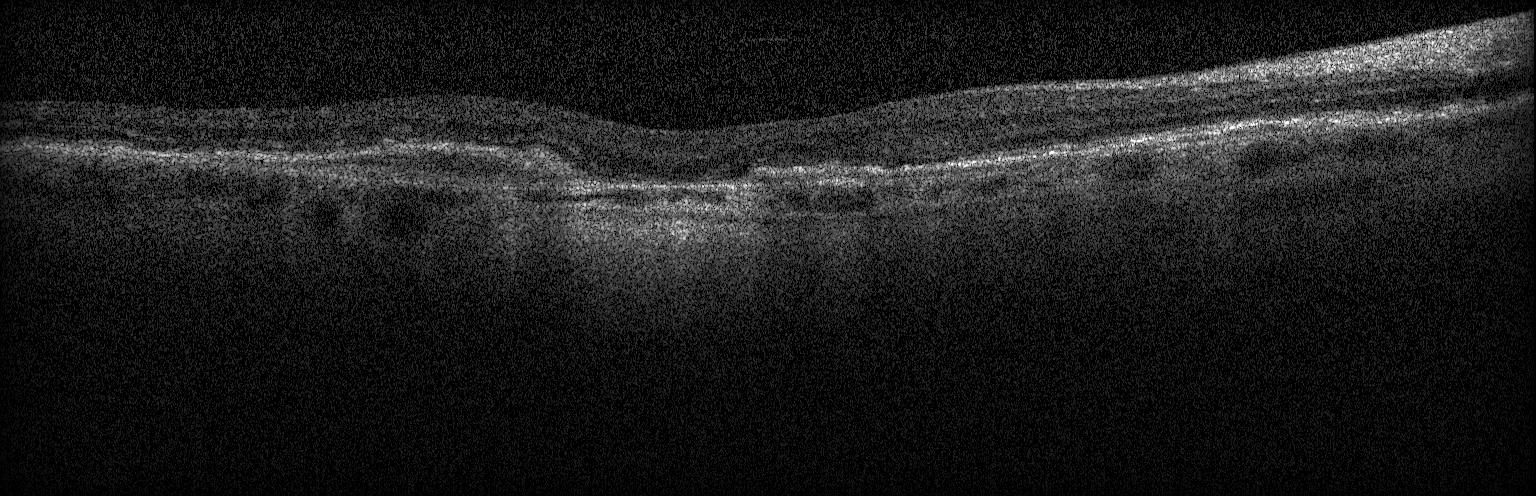

OCT line scan · Heidelberg Spectralis · horizontal scan through the fovea. This B-scan demonstrates a choroidal neovascular membrane.